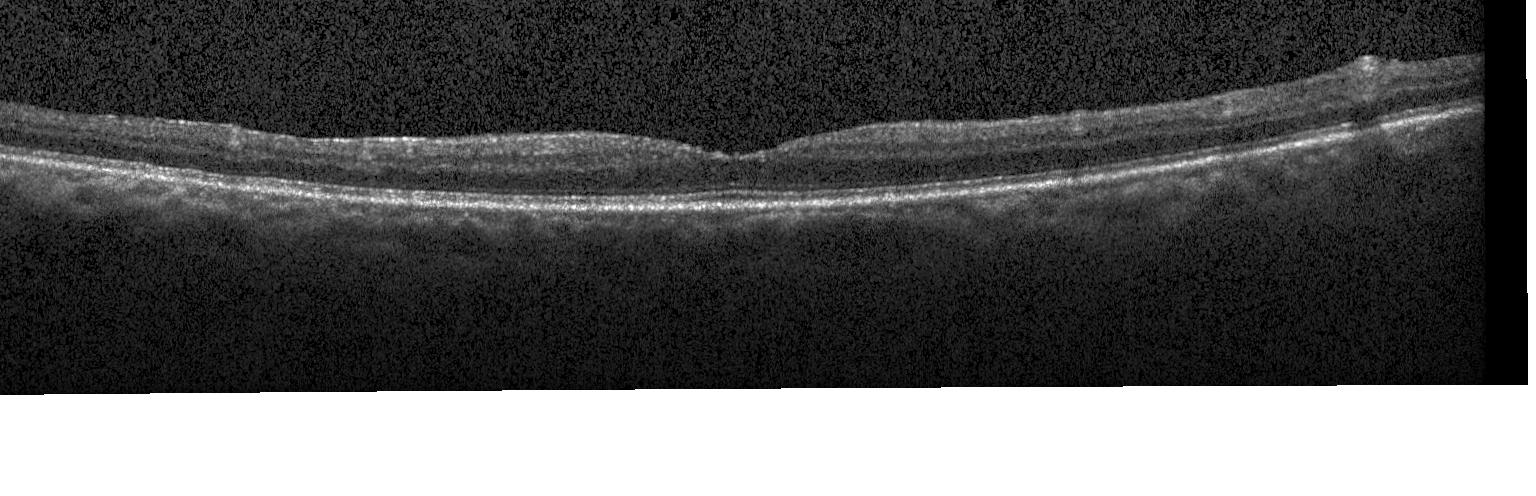

Optical coherence tomography scan — Diagnosis: no choroidal neovascularization, no diabetic macular edema, and no drusen.